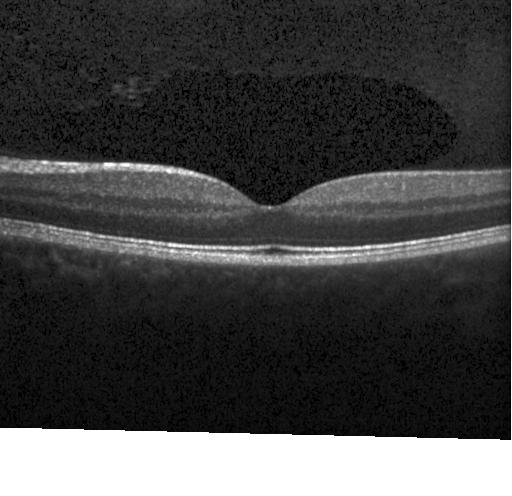
Optical coherence tomography scan
No evidence of CNV, DME, or drusen.